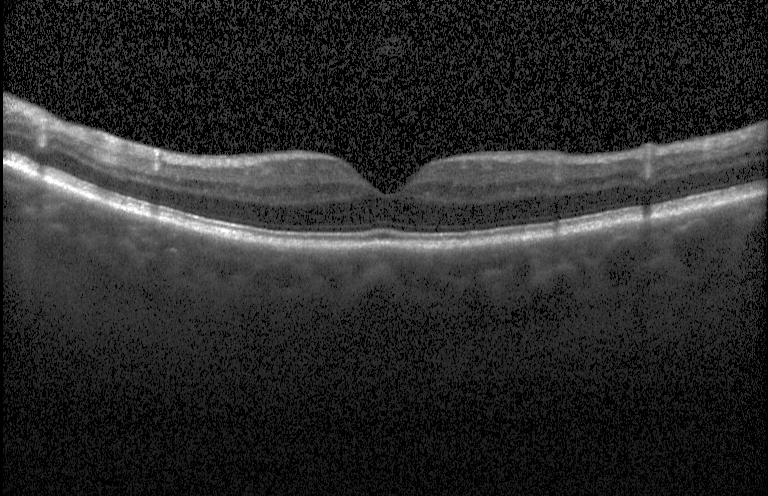

OCT B-scan — Impression: no evidence of choroidal neovascularization, diabetic macular edema, or drusen.